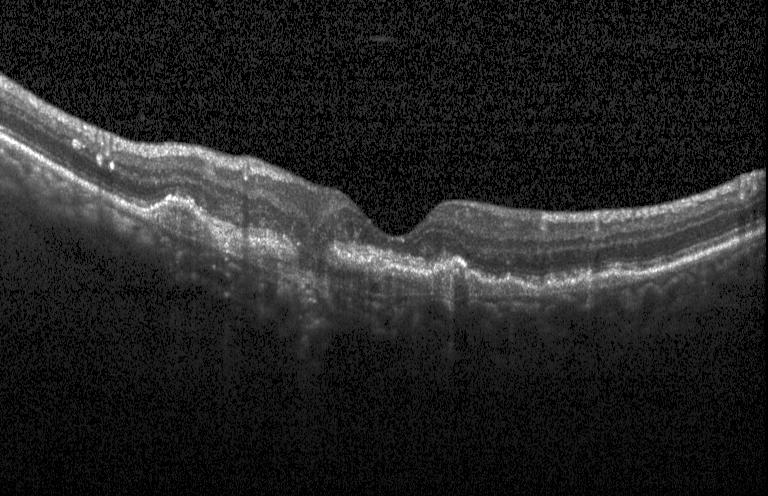
Macular OCT: a choroidal neovascular membrane.